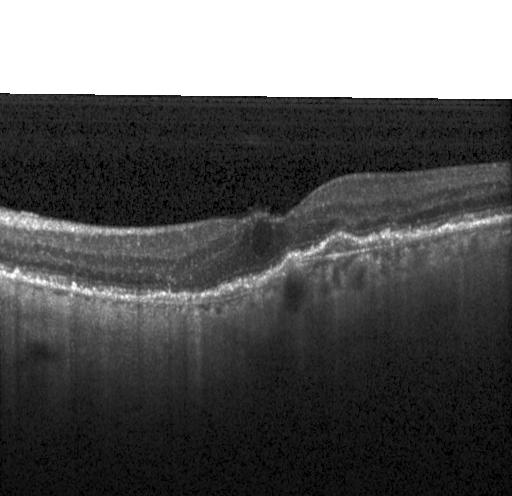
OCT B-scan showing a choroidal neovascular membrane.